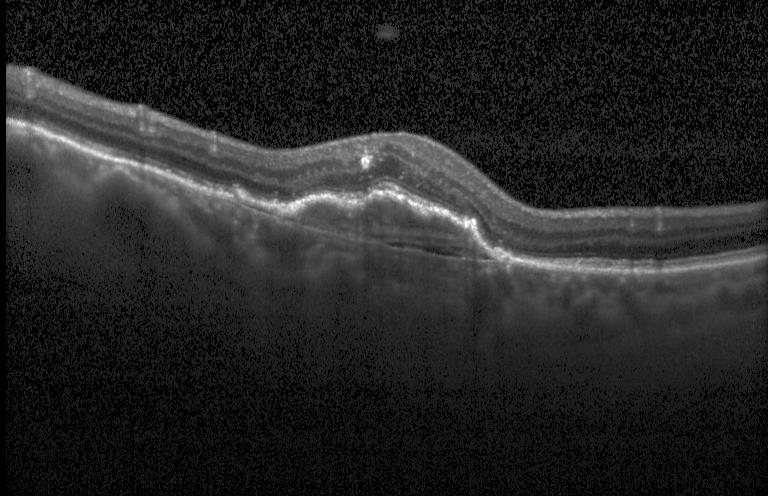 Diagnosis: choroidal neovascularization.